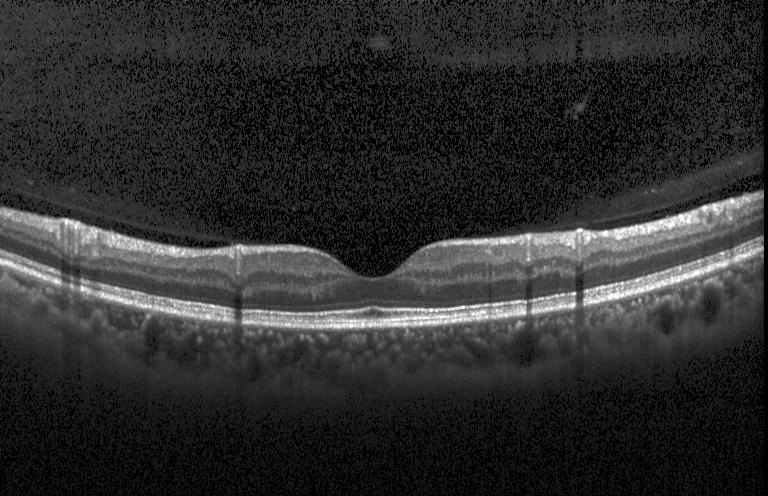 Retinal OCT B-scan.
This B-scan demonstrates no evidence of CNV, DME, or drusen.